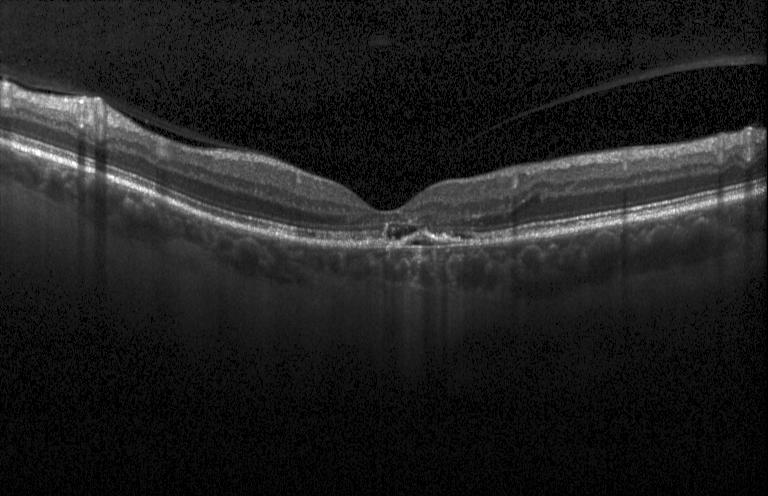
Retinal OCT B-scan · SD-OCT · centered on the fovea — Finding: a choroidal neovascular membrane.